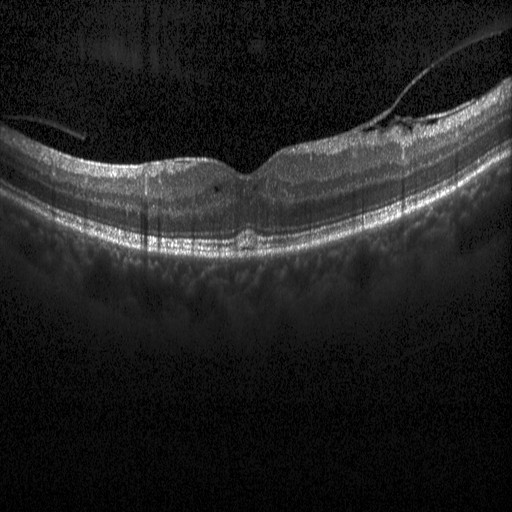

Spectral-domain optical coherence tomography, OCT line scan, Heidelberg Spectralis. DME.